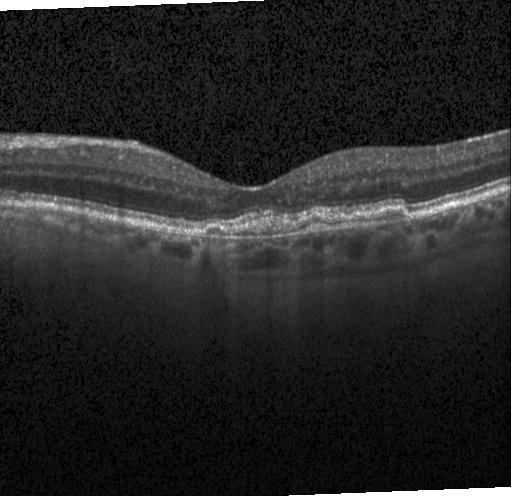 OCT scan showing choroidal neovascularization (CNV).